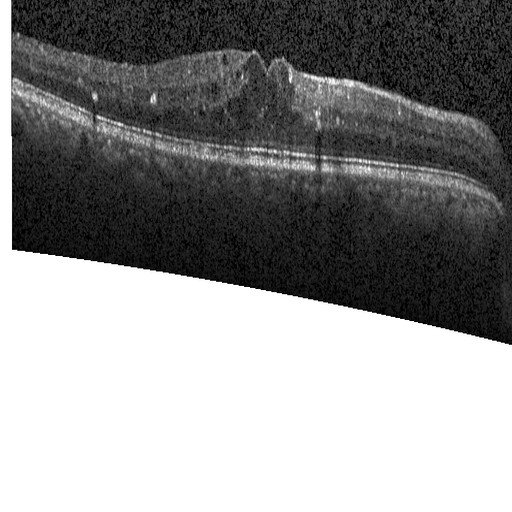
Macular OCT demonstrating diabetic macular edema.